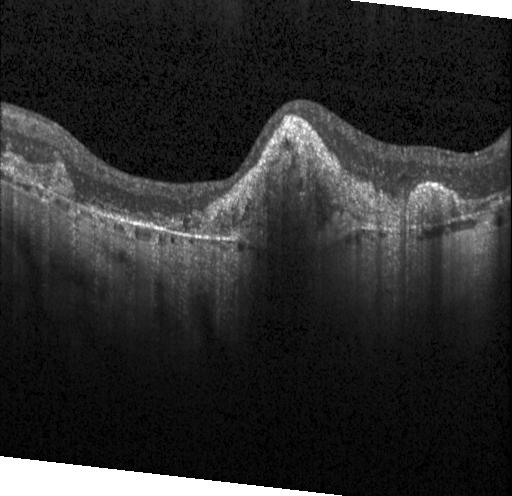
Optical coherence tomography B-scan · instrument: Heidelberg Spectralis · spectral-domain optical coherence tomography · horizontal scan through the fovea — CNV.